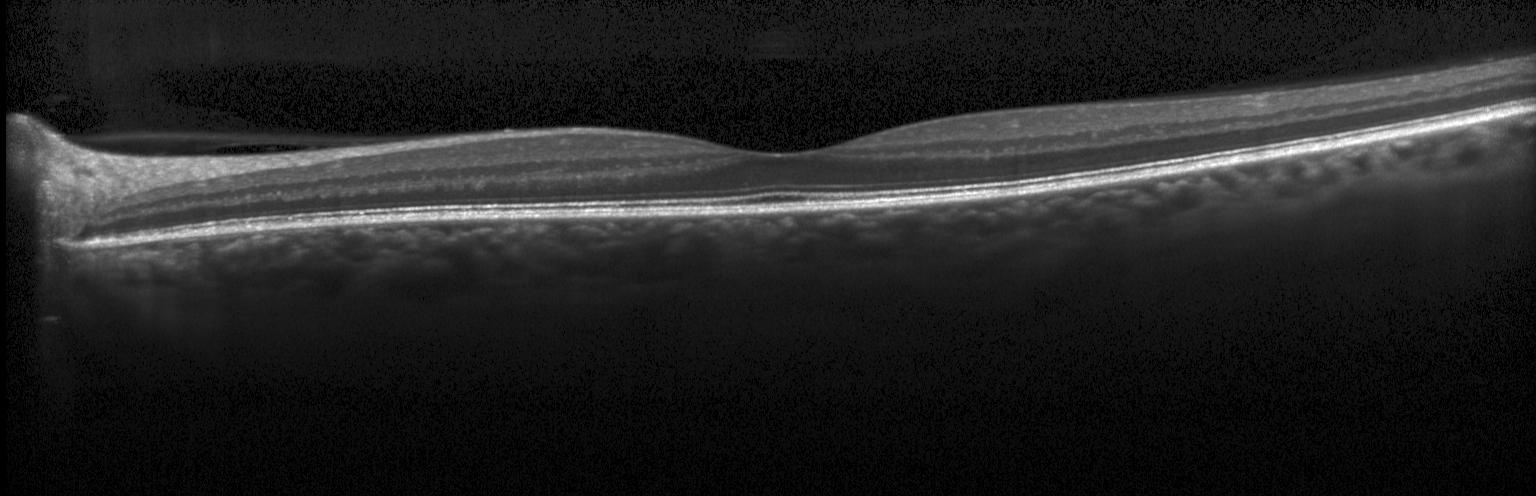
Through the macula, Heidelberg Spectralis, OCT line scan — Finding: no choroidal neovascularization, no diabetic macular edema, and no drusen.